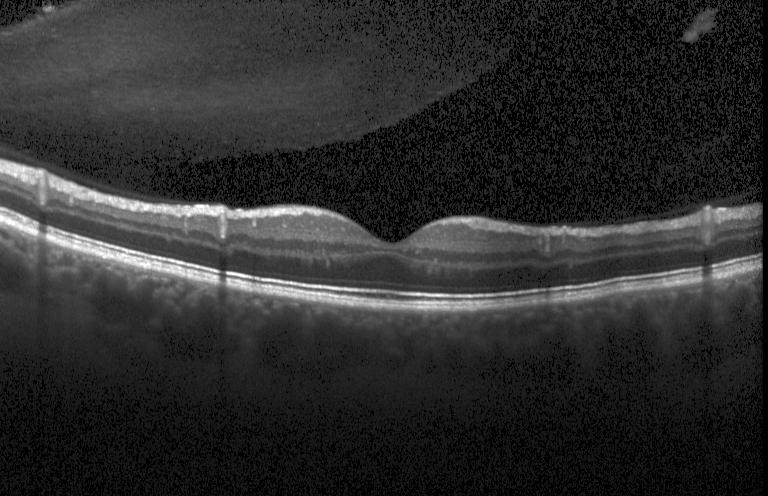 This B-scan demonstrates no choroidal neovascularization, no diabetic macular edema, and no drusen.